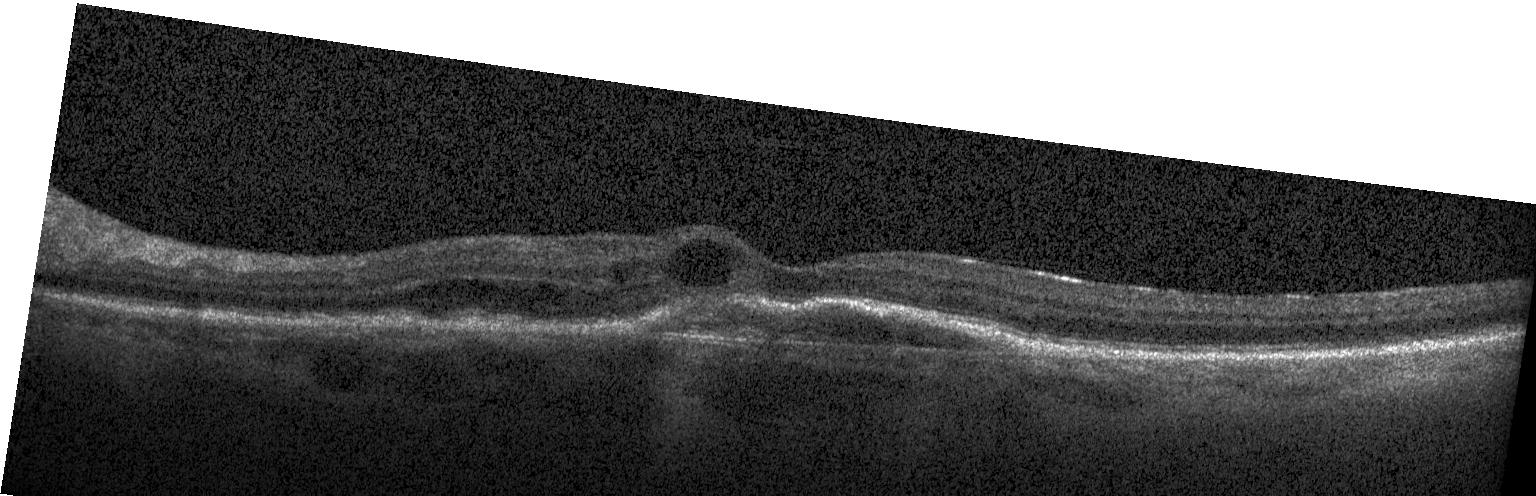

Macular OCT demonstrating a choroidal neovascular membrane.